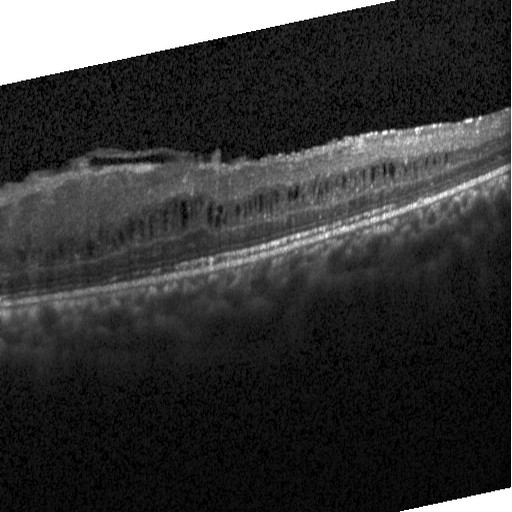 OCT line scan — Dx: DME.